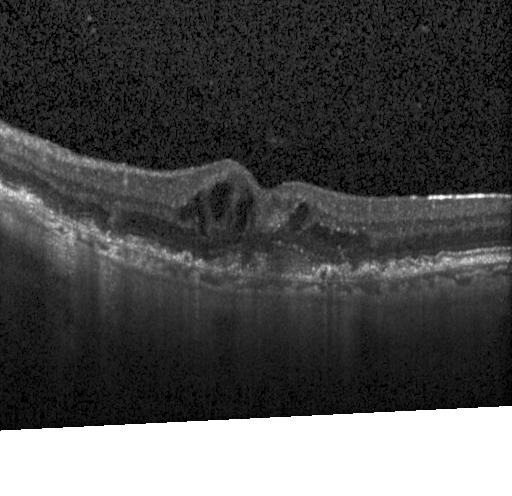 This B-scan demonstrates CNV.